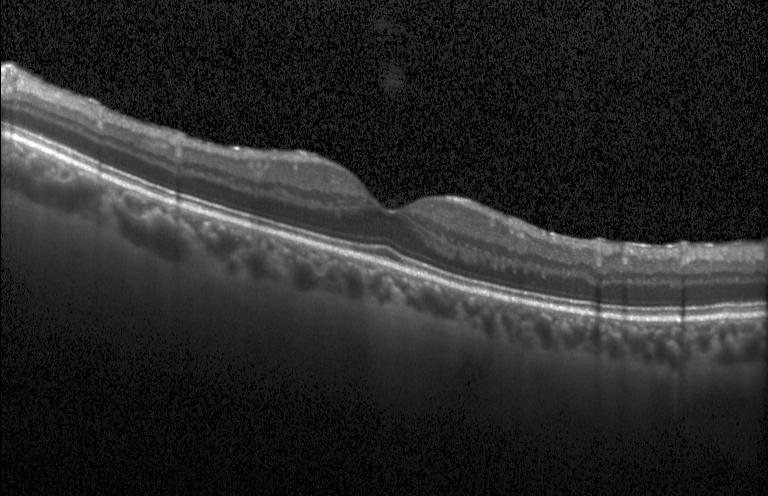 Horizontal scan through the fovea · optical coherence tomography scan · Heidelberg Spectralis · spectral-domain OCT. Macular OCT: neither choroidal neovascularization, diabetic macular edema, nor drusen.